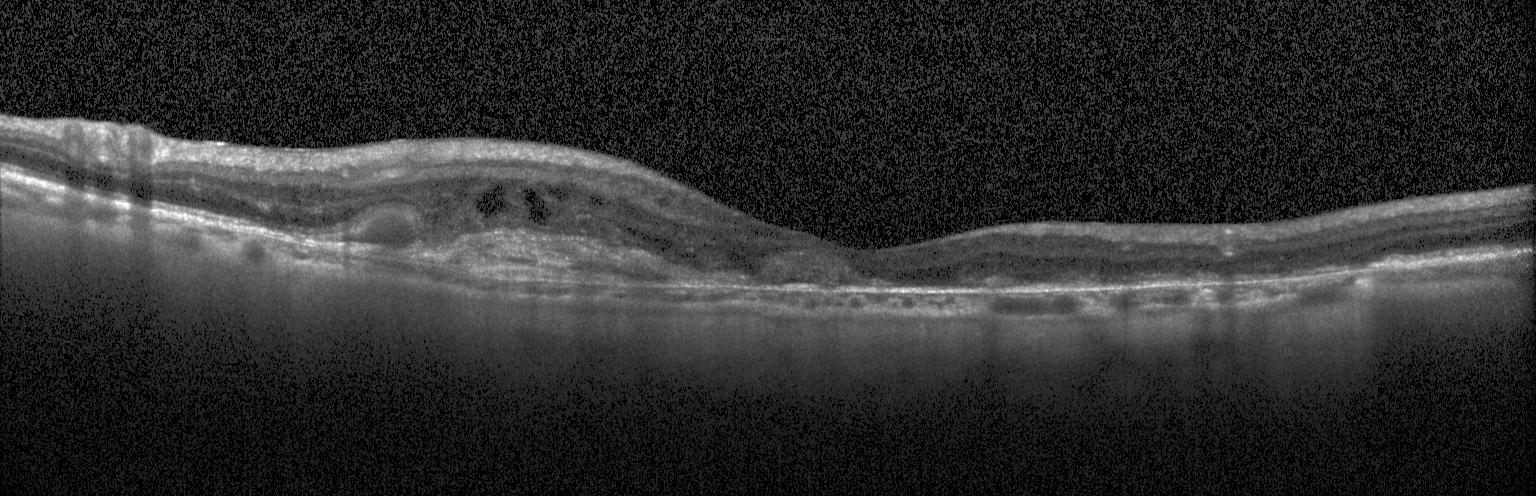
Retinal OCT cross-section, spectral-domain OCT. Diagnosis: choroidal neovascularization.